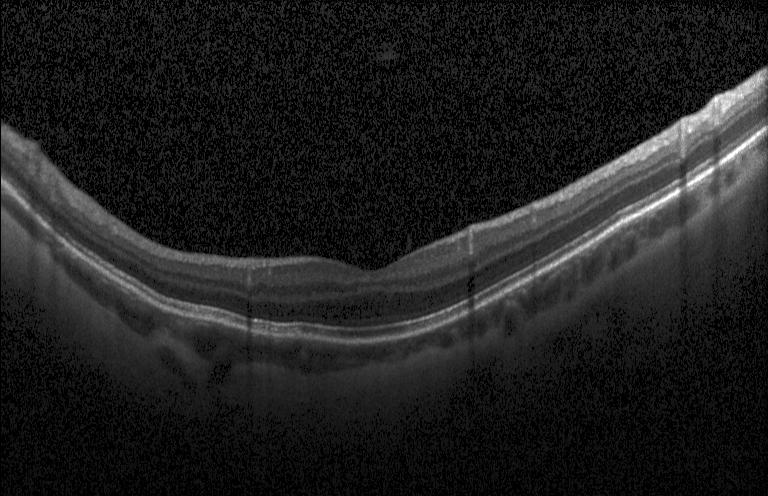

Assessment: neither CNV, DME, nor drusen.